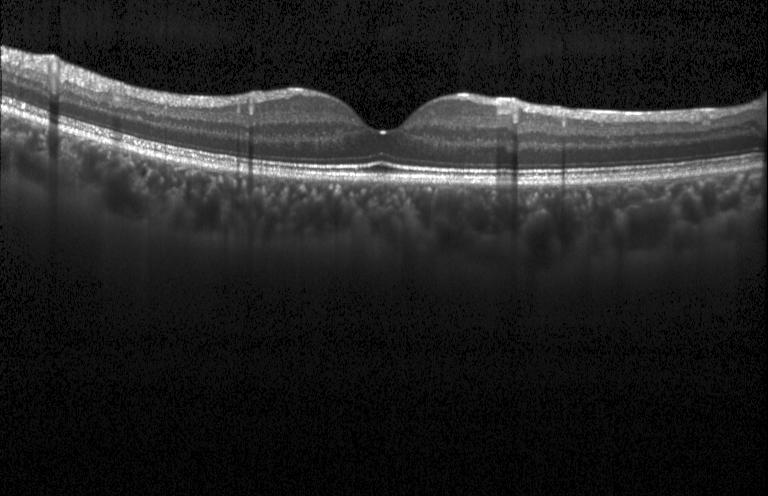
Retinal OCT cross-section showing no choroidal neovascularization, no diabetic macular edema, and no drusen.